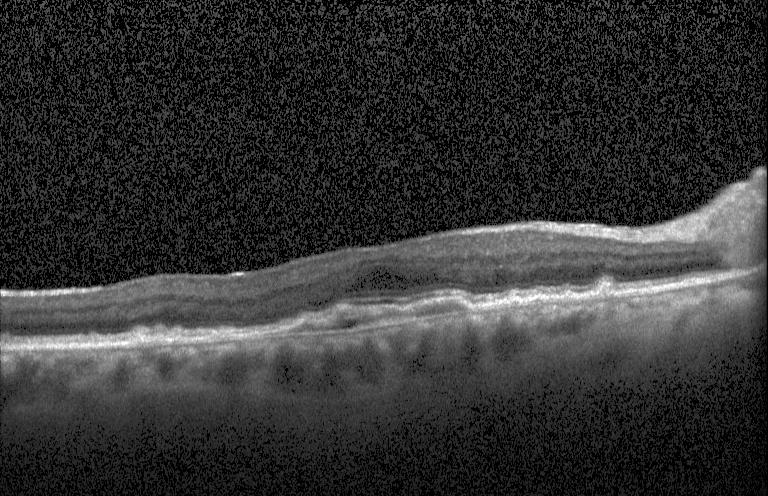

Fovea-centered · spectral-domain optical coherence tomography · Heidelberg Spectralis · OCT B-scan
Impression: choroidal neovascularization (CNV).